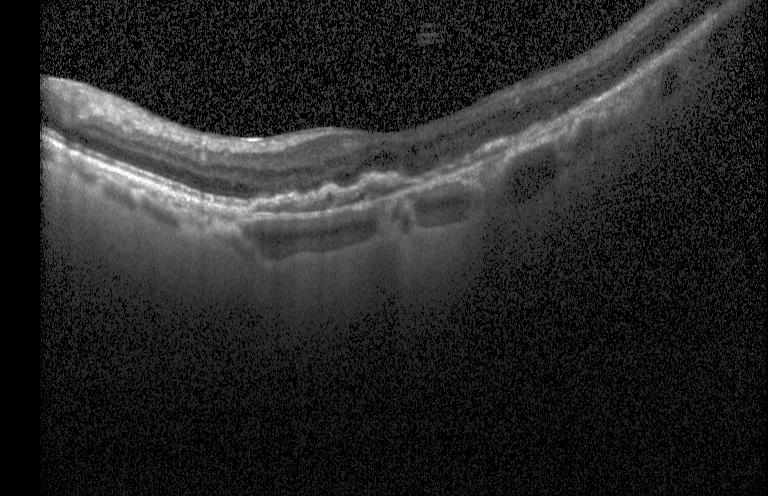
OCT B-scan · Heidelberg Spectralis OCT system · centered on the fovea · SD-OCT
OCT finding: CNV.